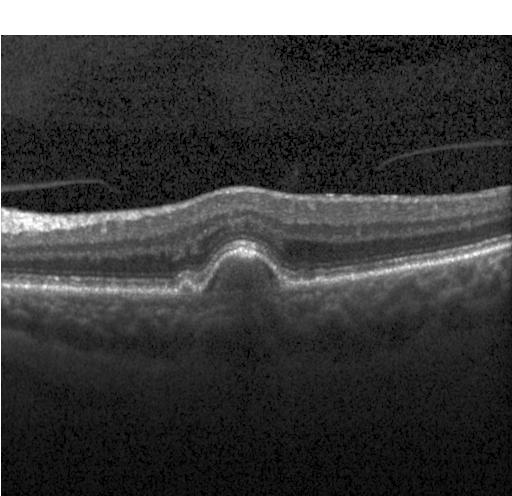

Through the macula. Optical coherence tomography scan
OCT finding: choroidal neovascularization.